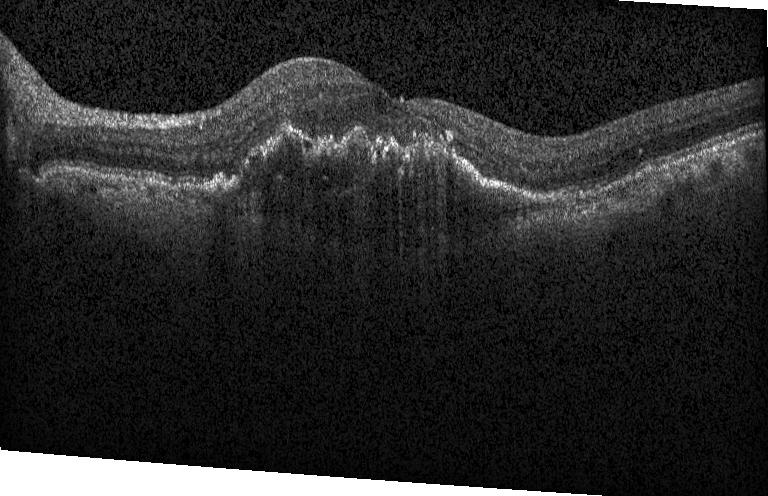

Optical coherence tomography scan. Spectral-domain OCT. Heidelberg Spectralis
Impression: a choroidal neovascular membrane.